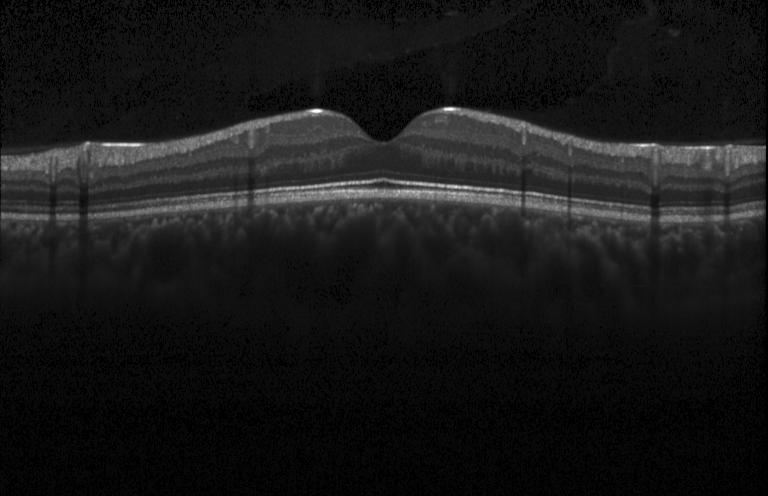

Fovea-centered; OCT B-scan.
Diagnosis: no evidence of CNV, DME, or drusen.